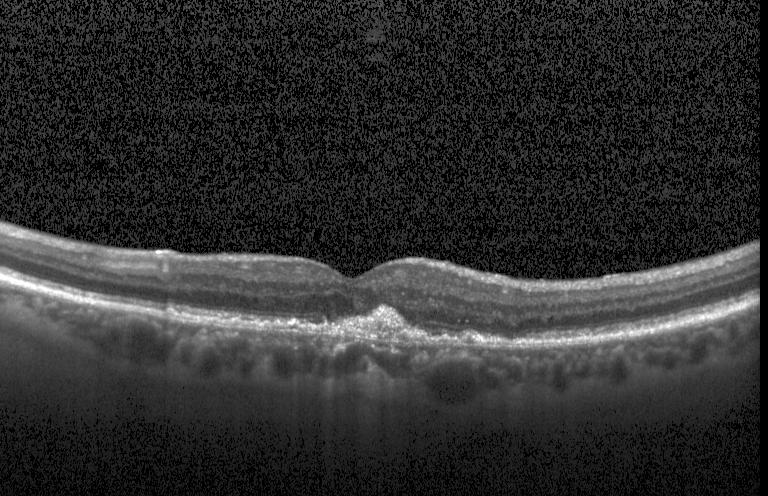
OCT scan showing a choroidal neovascular membrane.